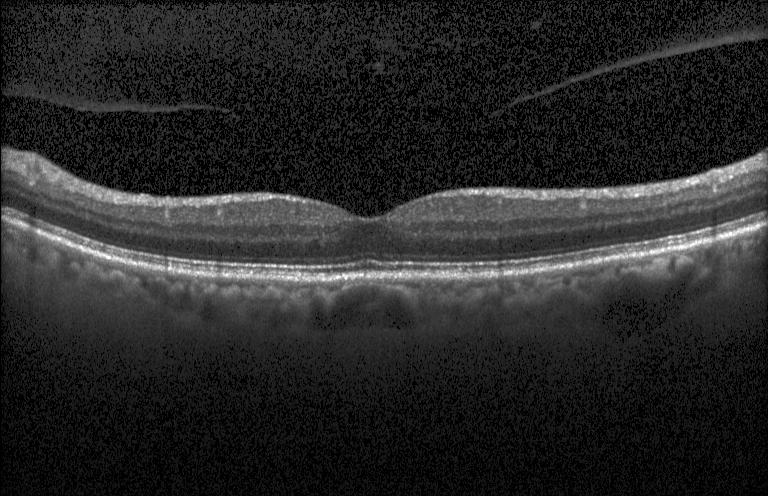

Assessment: neither choroidal neovascularization, diabetic macular edema, nor drusen.